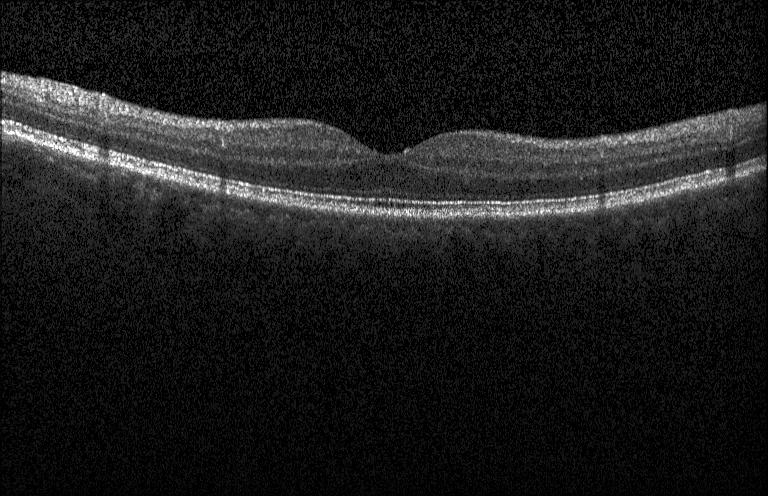 Through the macula · Heidelberg Spectralis · retinal OCT cross-section · spectral-domain optical coherence tomography — Macular OCT: no choroidal neovascularization, diabetic macular edema, or drusen.